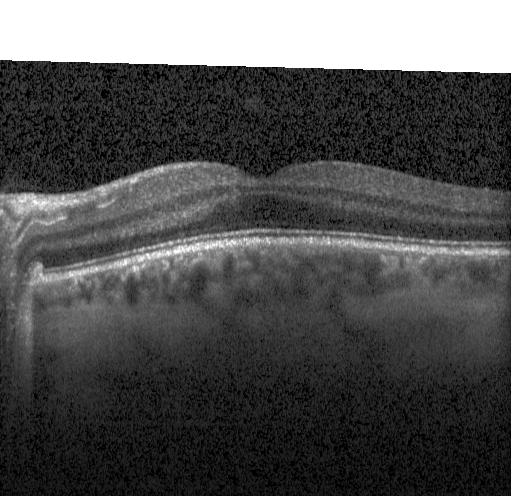
Impression: no choroidal neovascularization, no diabetic macular edema, and no drusen.